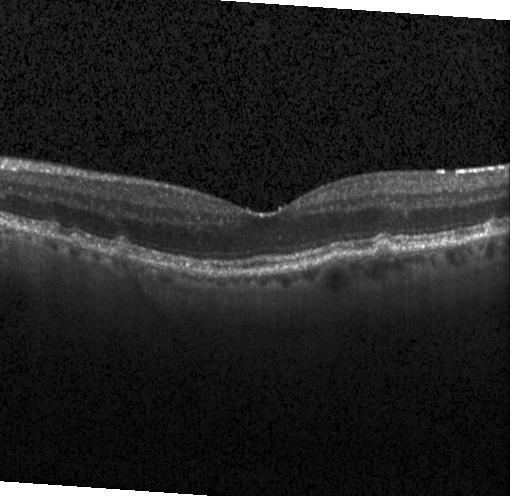 This B-scan demonstrates drusen.